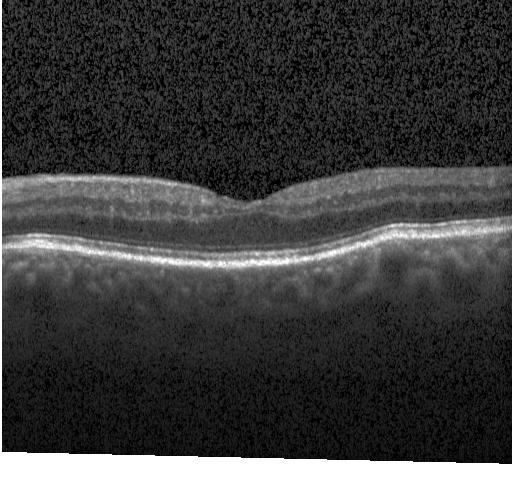 Macular OCT: no CNV, DME, or drusen.